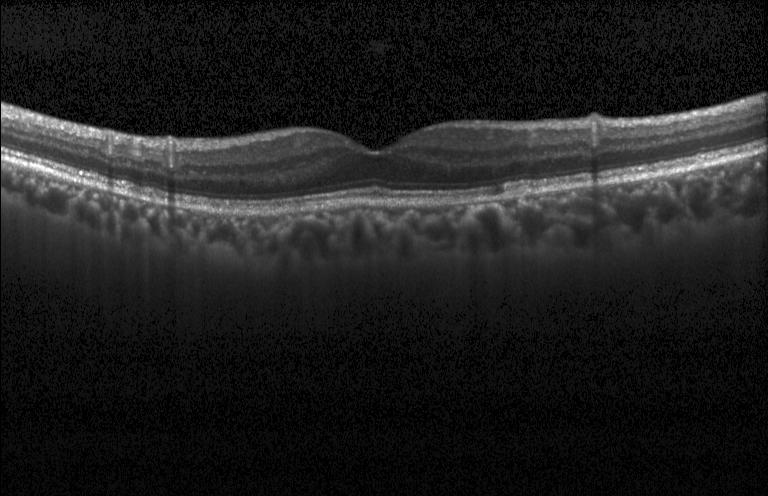
Finding: neither choroidal neovascularization, diabetic macular edema, nor drusen.